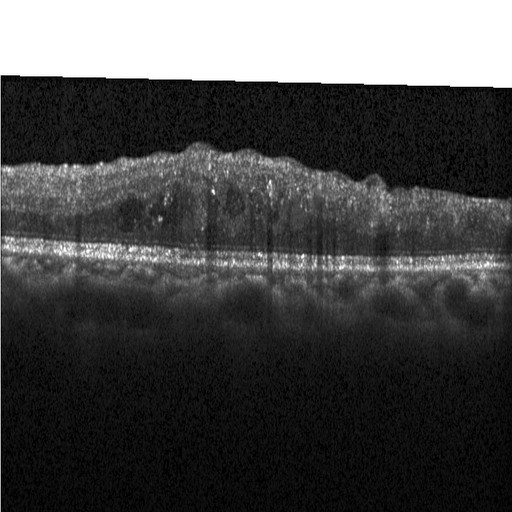

The scan shows DME.